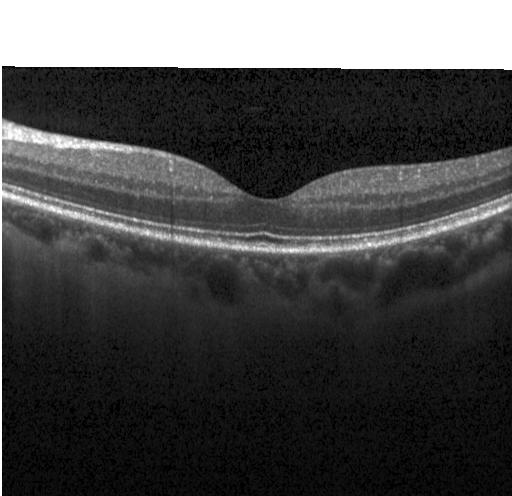 Horizontal scan through the fovea · Heidelberg Spectralis · spectral-domain OCT · retinal OCT cross-section
The scan shows no choroidal neovascularization, diabetic macular edema, or drusen.